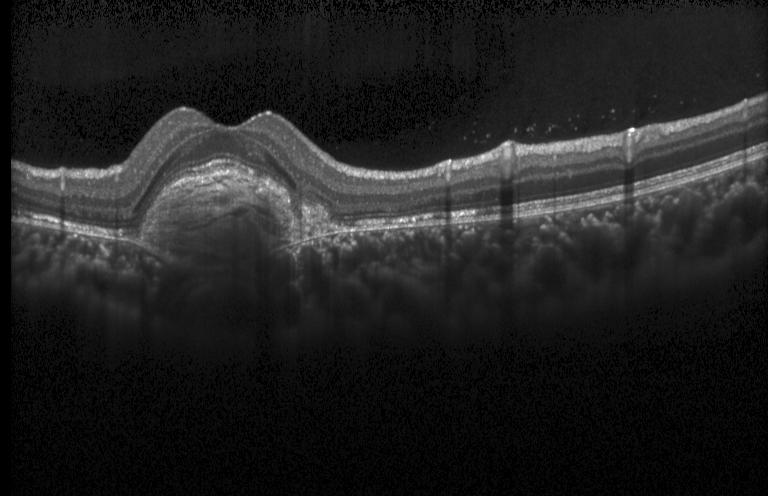

Diagnosis: choroidal neovascularization.